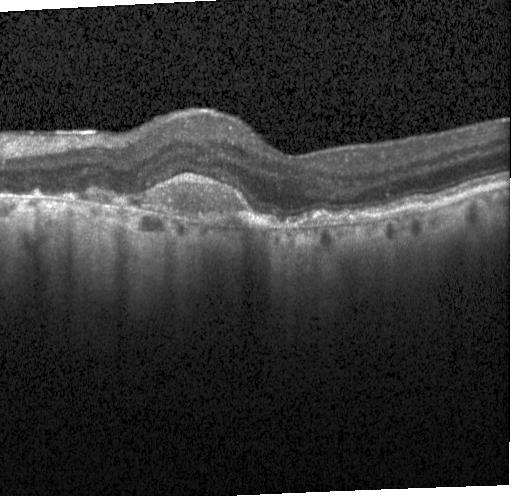

Retinal OCT cross-section
OCT finding: a choroidal neovascular membrane.